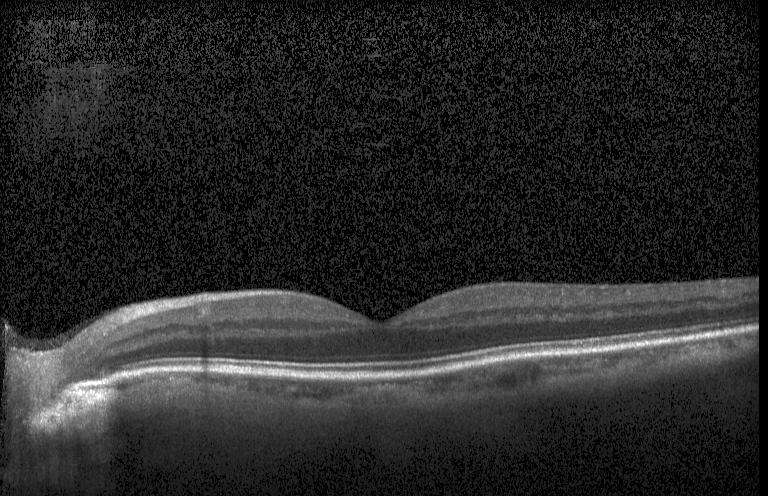 SD-OCT. Retinal OCT B-scan. Fovea-centered
This B-scan demonstrates no evidence of choroidal neovascularization, diabetic macular edema, or drusen.